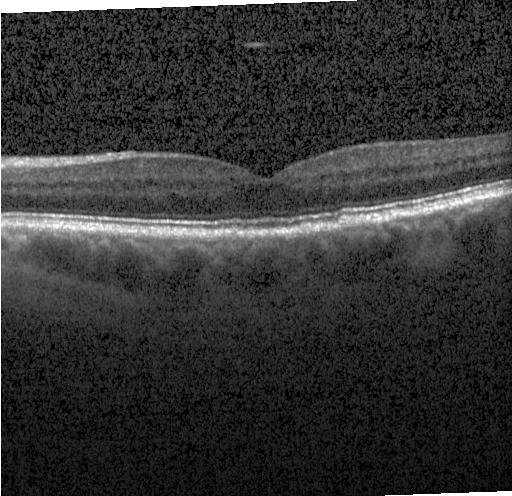

OCT finding: multiple drusen.